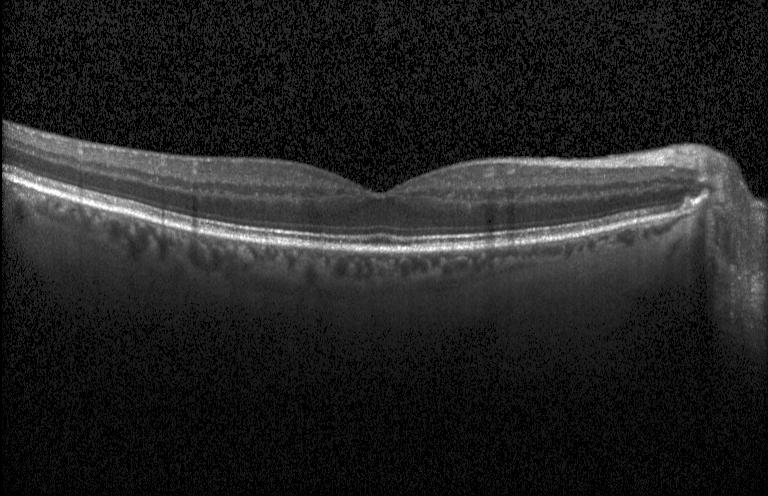
Impression: neither CNV, DME, nor drusen.